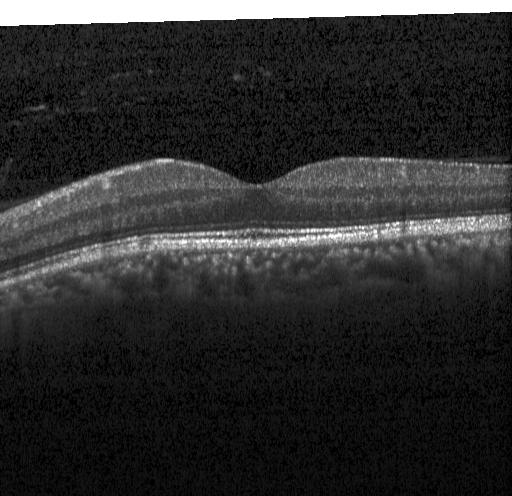

Heidelberg Spectralis OCT system, SD-OCT, fovea-centered, retinal OCT B-scan — Assessment: neither CNV, DME, nor drusen.